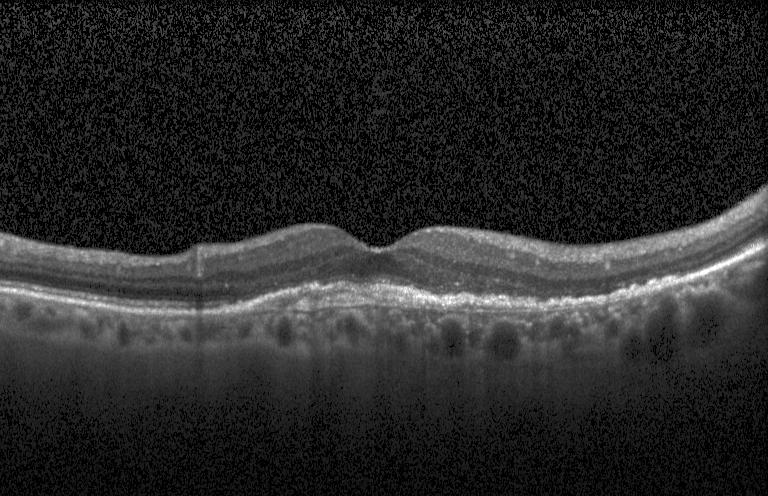 Optical coherence tomography scan.
OCT finding: CNV.